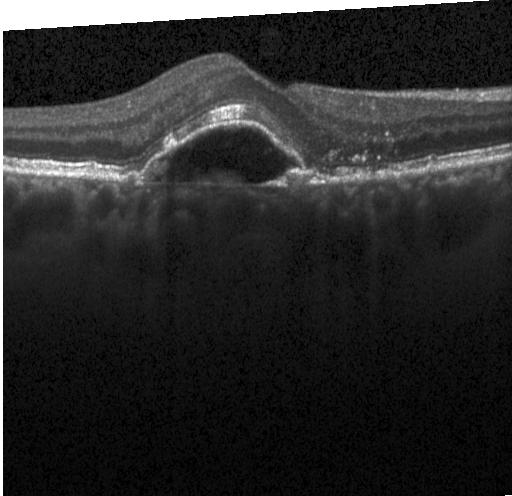

Impression: choroidal neovascularization.